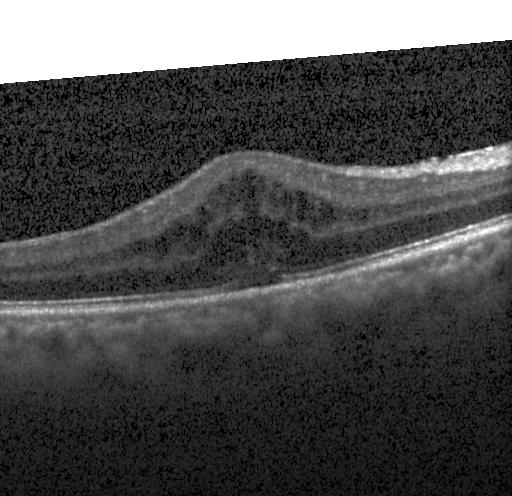

OCT line scan, acquired on a Heidelberg Spectralis, spectral-domain OCT, horizontal scan through the fovea. Finding: DME.